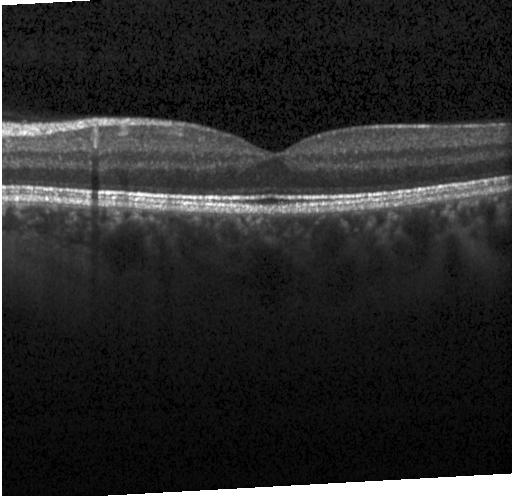
Through the macula; Heidelberg Spectralis OCT system; spectral-domain OCT; retinal OCT B-scan
Finding: no choroidal neovascularization, diabetic macular edema, or drusen.